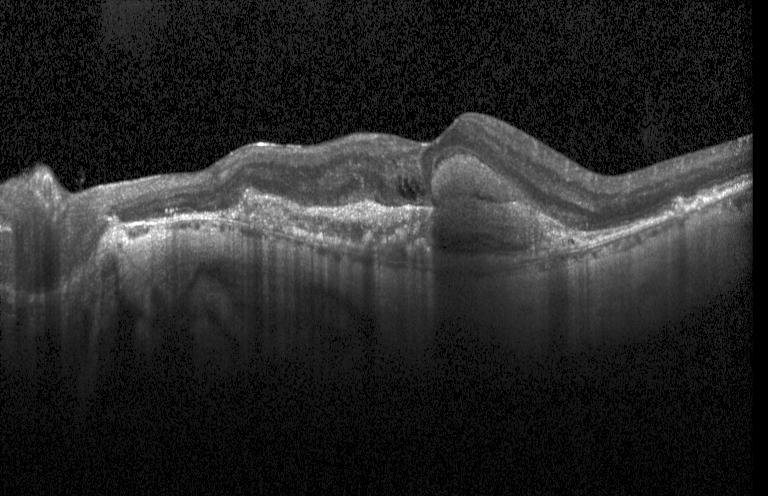

Impression: a choroidal neovascular membrane.